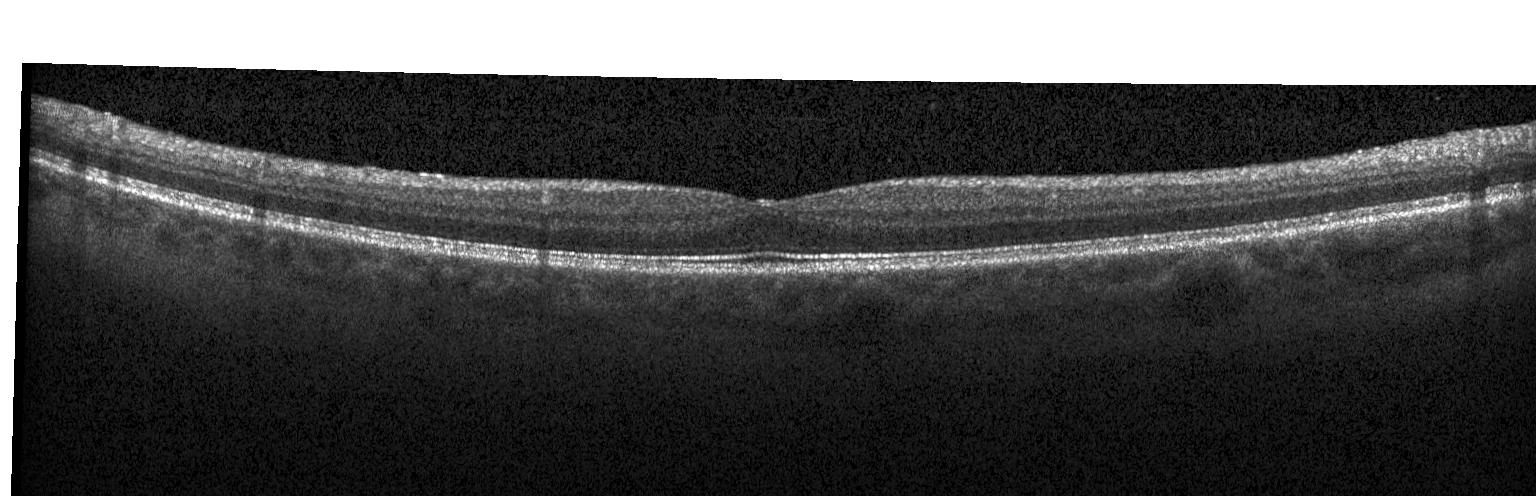

Retinal OCT cross-section; spectral-domain optical coherence tomography; acquired on a Heidelberg Spectralis. Finding: no choroidal neovascularization, no diabetic macular edema, and no drusen.